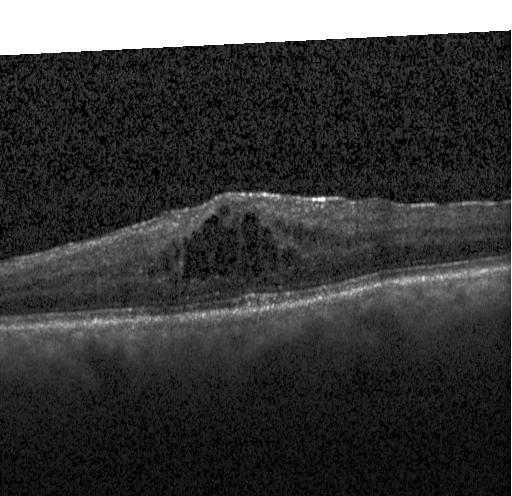
Impression: diabetic macular edema (DME).